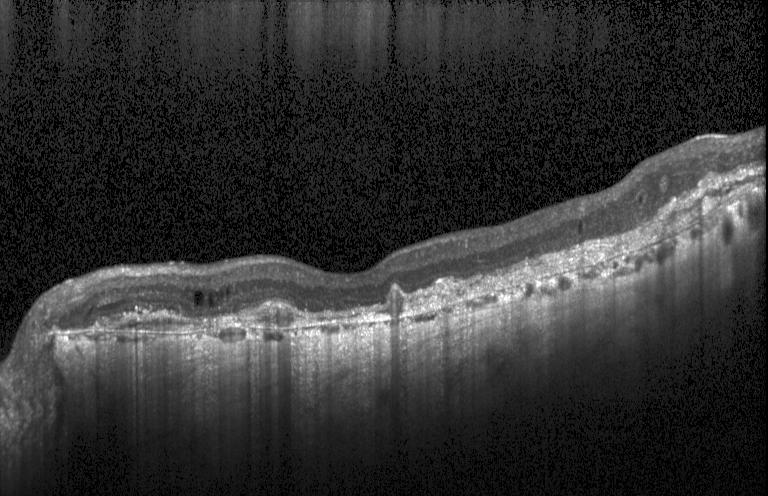

Optical coherence tomography B-scan · SD-OCT — The scan shows choroidal neovascularization.